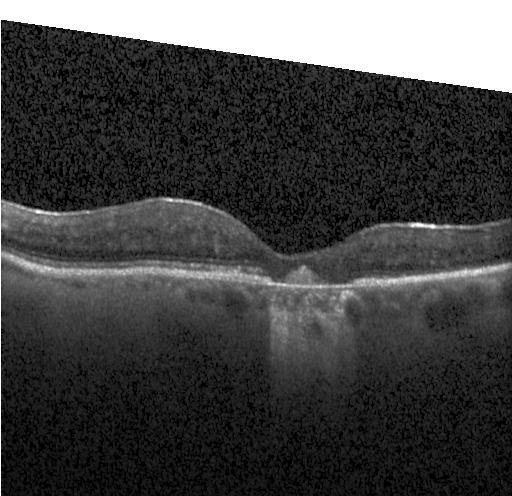 Fovea-centered; SD-OCT; OCT line scan
OCT finding: CNV.